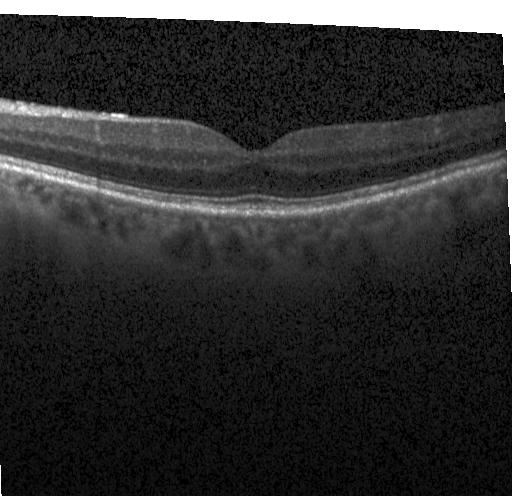 Dx: no choroidal neovascularization, diabetic macular edema, or drusen.